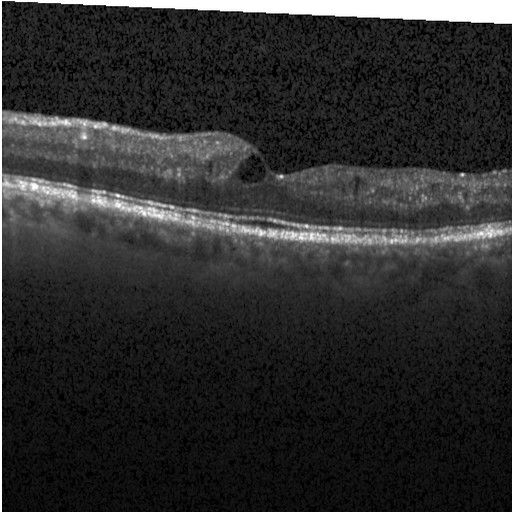
Horizontal scan through the fovea · instrument: Heidelberg Spectralis · optical coherence tomography scan · spectral-domain OCT — Impression: diabetic macular edema.